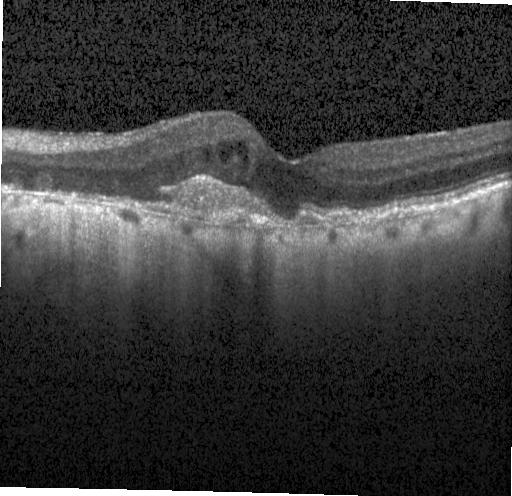 This B-scan demonstrates a choroidal neovascular membrane.